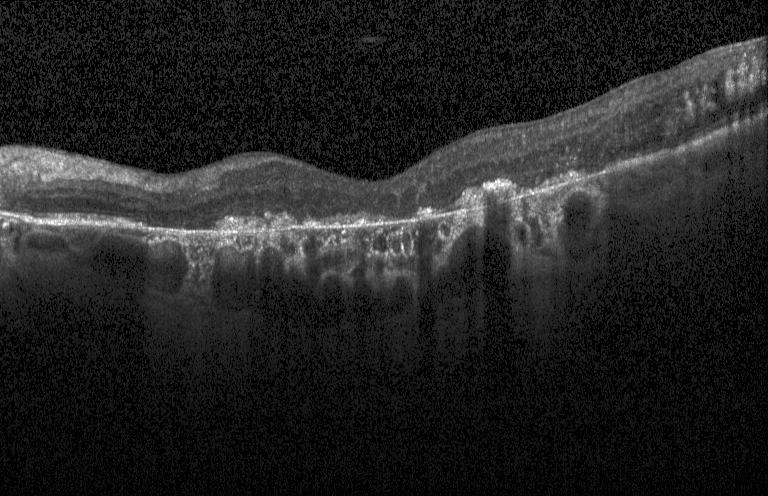
This B-scan demonstrates a choroidal neovascular membrane.